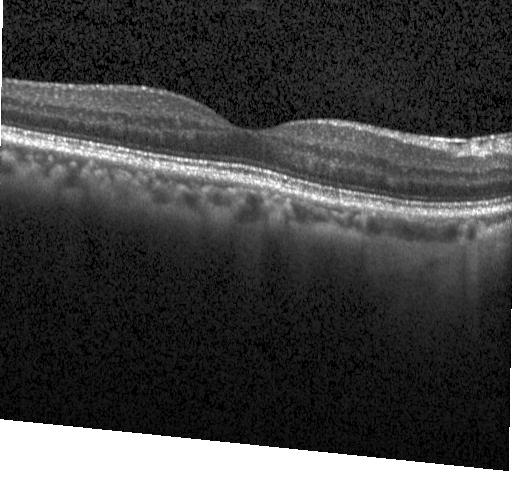

Spectral-domain OCT · horizontal scan through the fovea · optical coherence tomography B-scan · Heidelberg Spectralis OCT system — Assessment: neither choroidal neovascularization, diabetic macular edema, nor drusen.